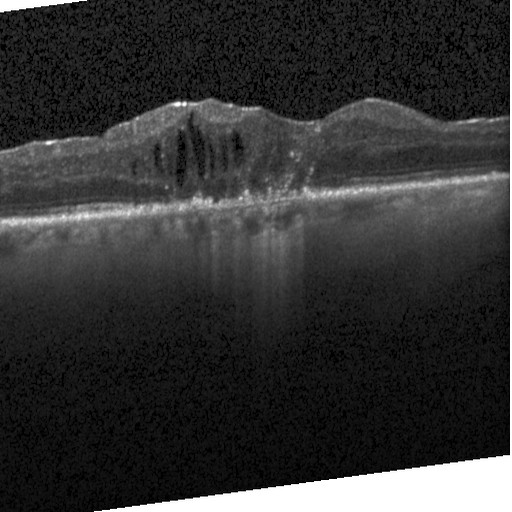

Impression: diabetic macular edema.